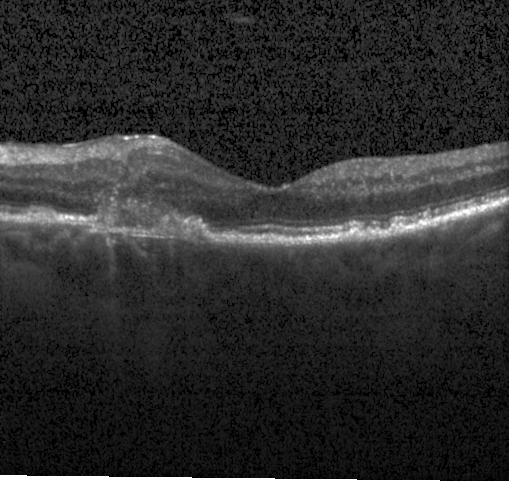
OCT finding: choroidal neovascularization (CNV).